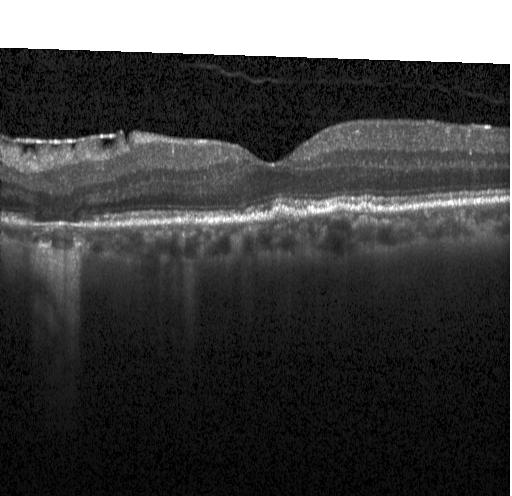

Finding: multiple drusen.